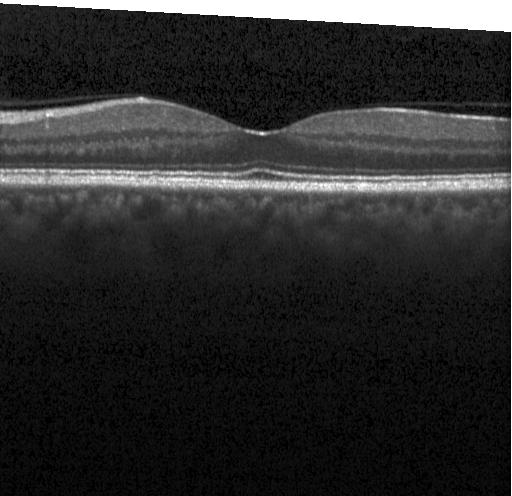
Retinal OCT B-scan. Horizontal scan through the fovea. Heidelberg Spectralis OCT system
Diagnosis: no choroidal neovascularization, diabetic macular edema, or drusen.